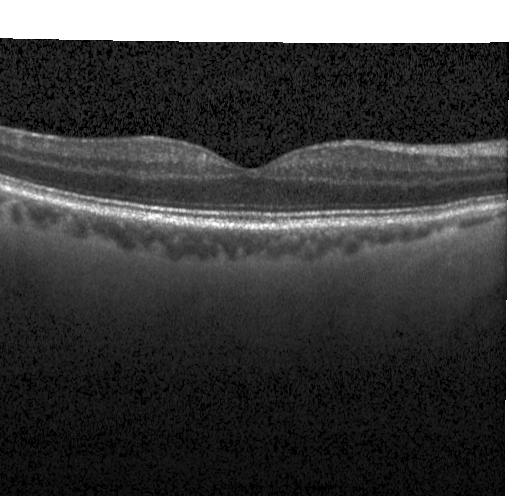
Optical coherence tomography scan. Heidelberg Spectralis — Assessment: no evidence of choroidal neovascularization, diabetic macular edema, or drusen.